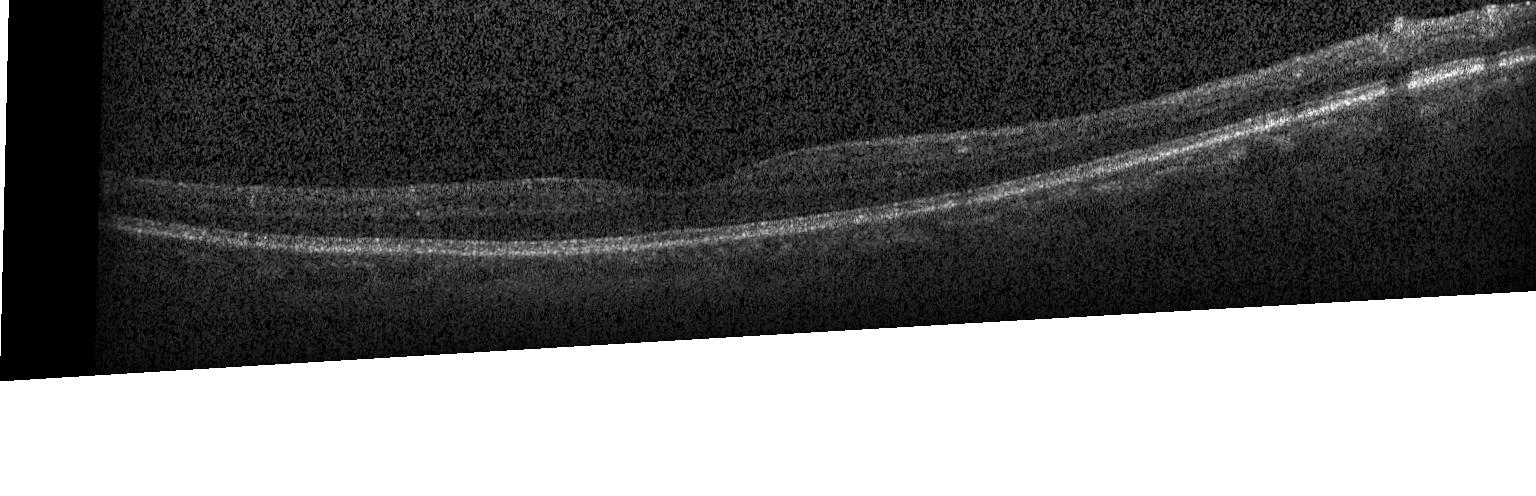
Horizontal scan through the fovea; optical coherence tomography B-scan.
No choroidal neovascularization, no diabetic macular edema, and no drusen.